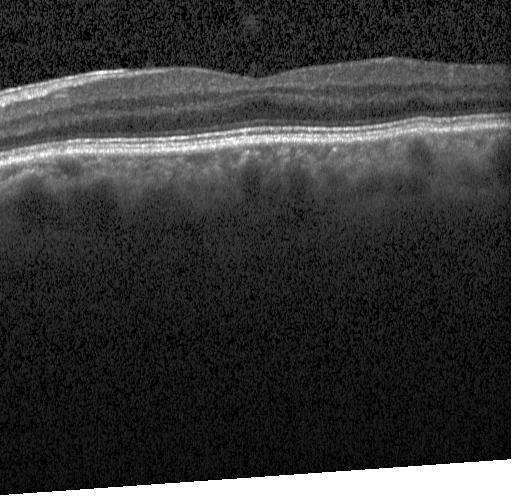
Macular OCT: no evidence of choroidal neovascularization, diabetic macular edema, or drusen.